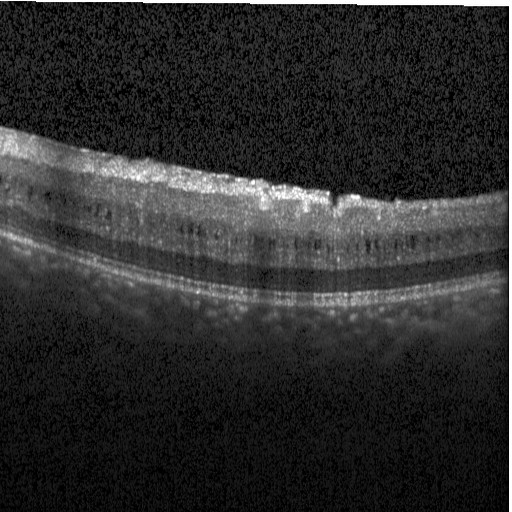
Finding: diabetic macular edema (DME).